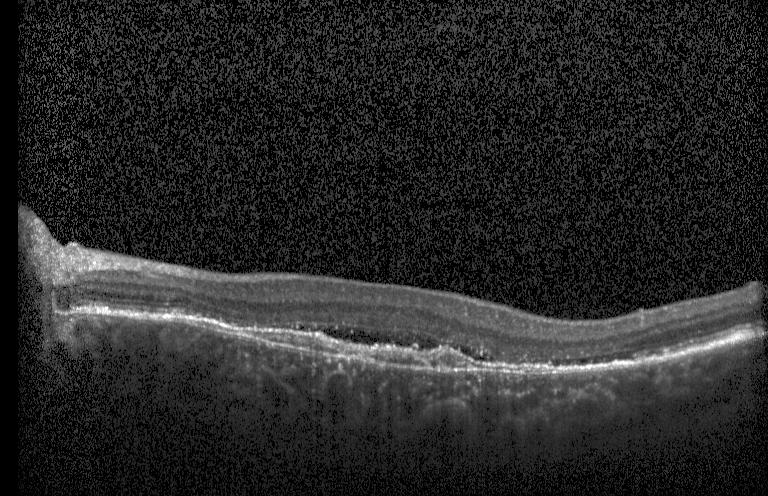
CNV.